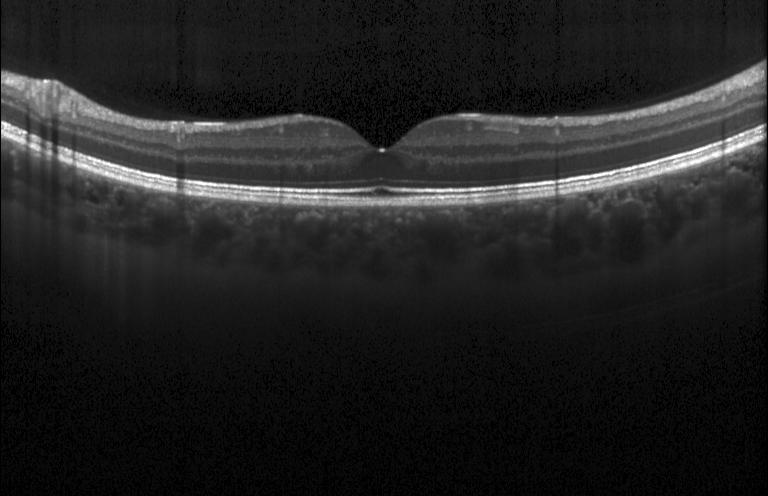

Retinal OCT cross-section showing no evidence of choroidal neovascularization, diabetic macular edema, or drusen.